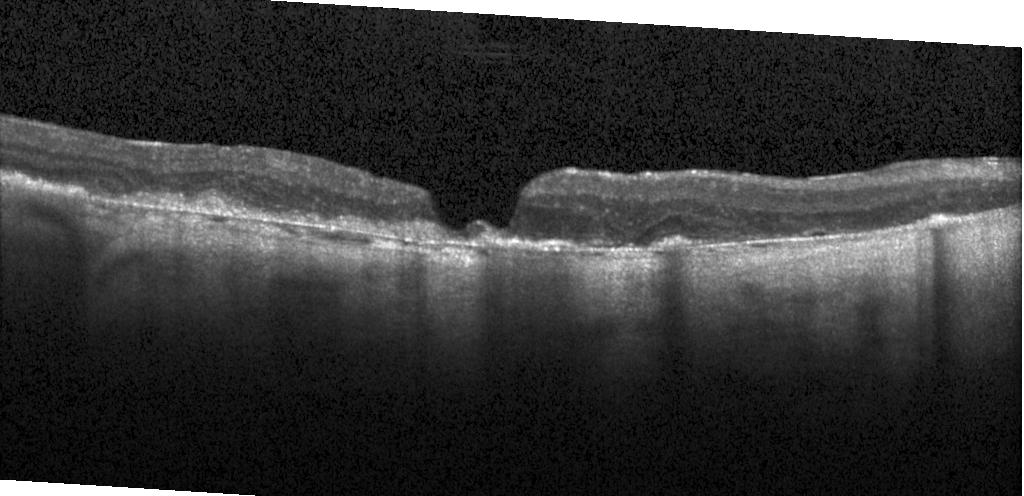 Optical coherence tomography scan. Spectral-domain optical coherence tomography.
The scan shows a choroidal neovascular membrane.